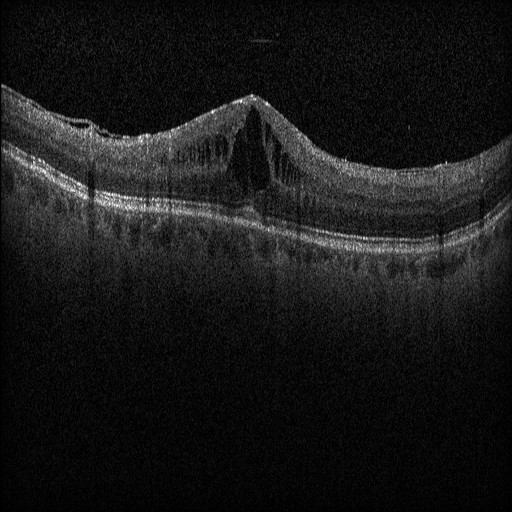
Retinal OCT B-scan.
Finding: DME.